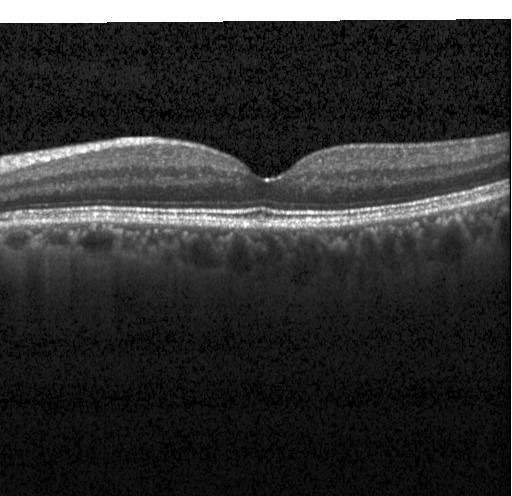
Neither CNV, DME, nor drusen.